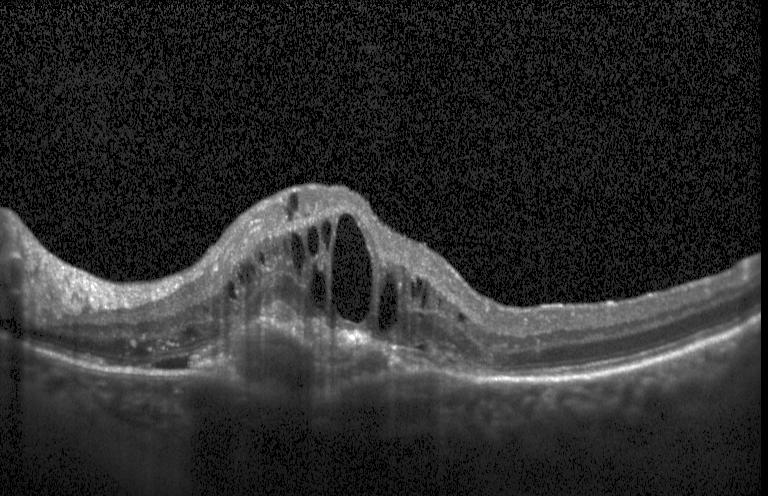 Macular scan; retinal OCT B-scan. Assessment: choroidal neovascularization.